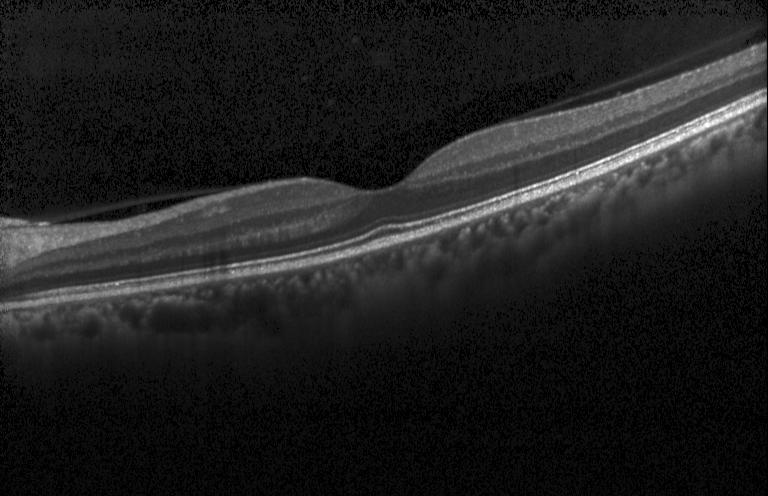 Macular OCT: no evidence of choroidal neovascularization, diabetic macular edema, or drusen.